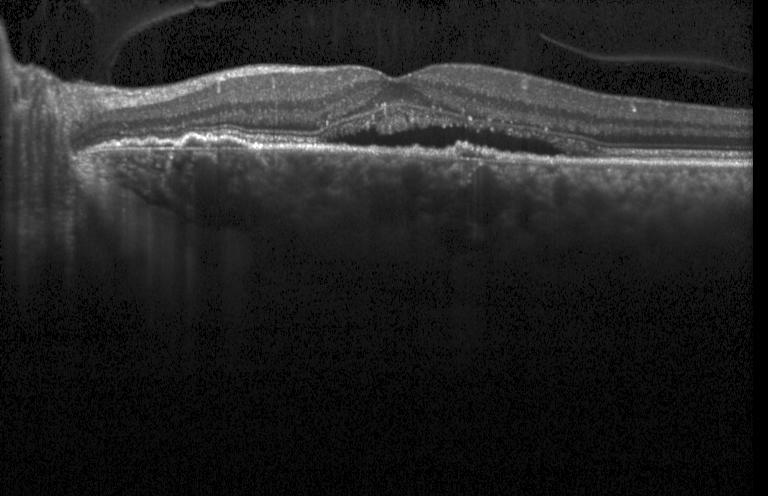
Horizontal scan through the fovea, Heidelberg Spectralis, retinal OCT cross-section, spectral-domain optical coherence tomography. Diagnosis: a choroidal neovascular membrane.